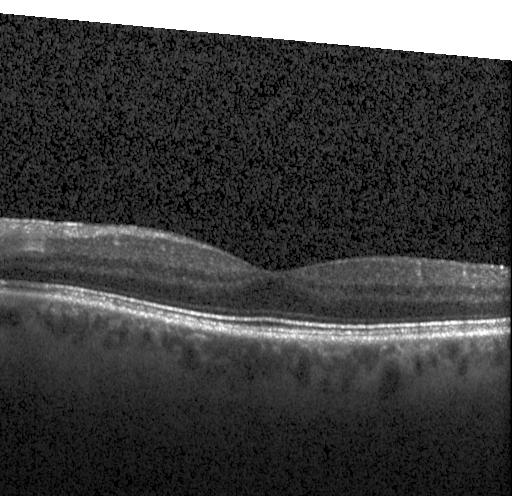
Retinal OCT cross-section. Impression: no choroidal neovascularization, diabetic macular edema, or drusen.